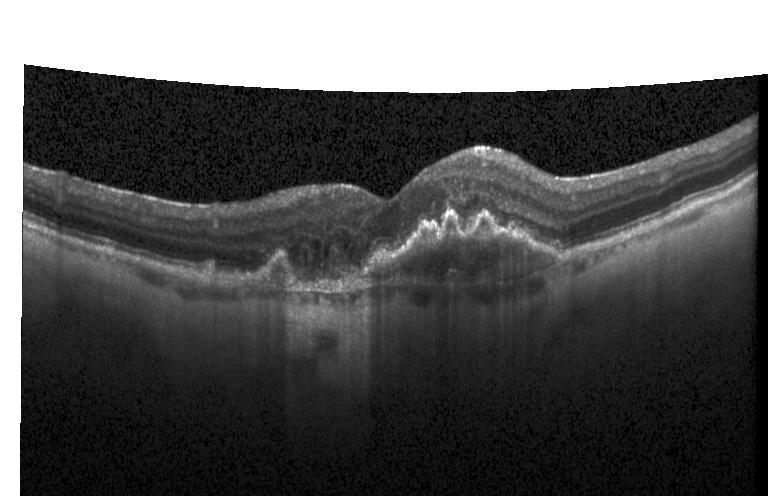

OCT B-scan · spectral-domain OCT.
Finding: a choroidal neovascular membrane.